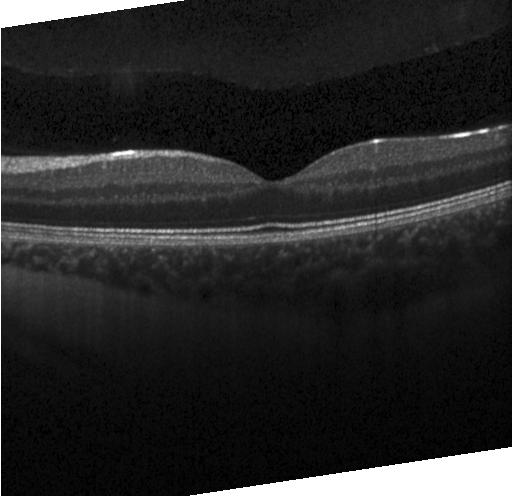
Retinal OCT cross-section
Assessment: no evidence of choroidal neovascularization, diabetic macular edema, or drusen.